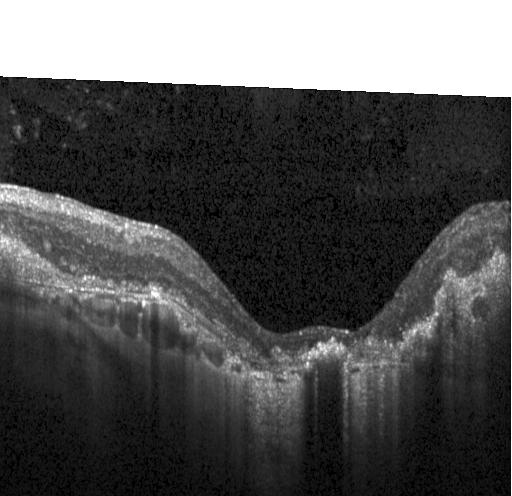

Optical coherence tomography B-scan, through the macula
Macular OCT: a choroidal neovascular membrane.